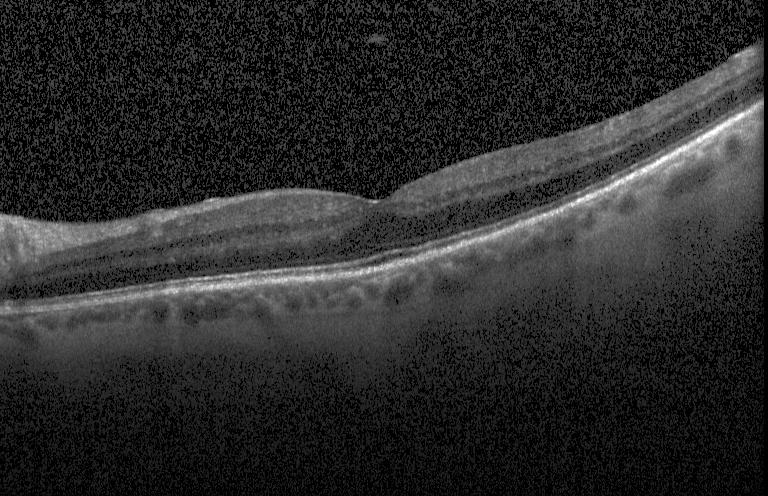 Centered on the fovea, acquired on a Heidelberg Spectralis, retinal OCT cross-section. The scan shows neither choroidal neovascularization, diabetic macular edema, nor drusen.